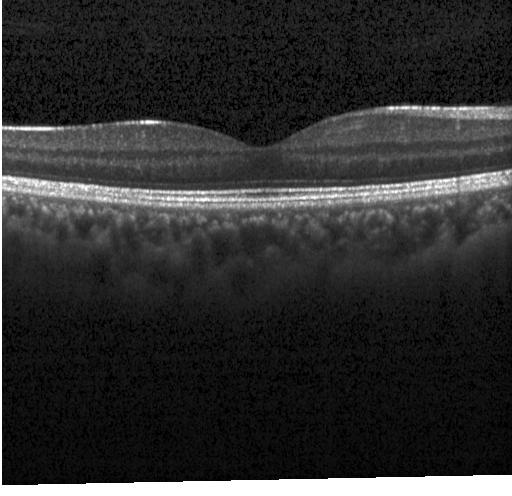 Macular OCT demonstrating neither choroidal neovascularization, diabetic macular edema, nor drusen.